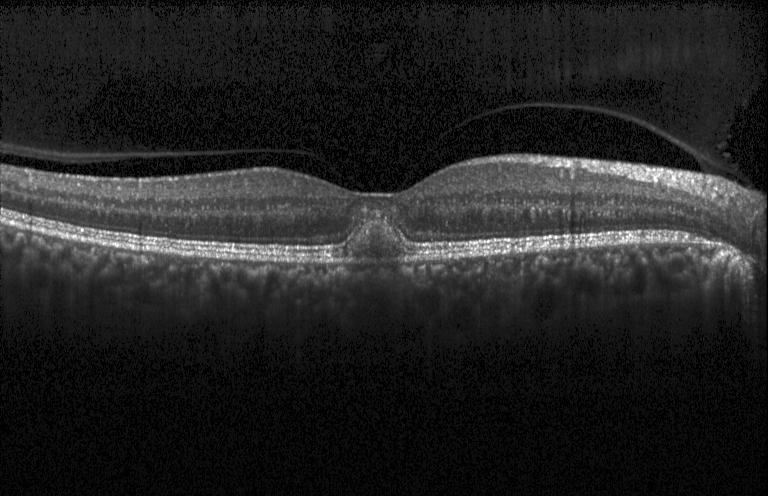

Retinal OCT B-scan — Diagnosis: choroidal neovascularization (CNV).